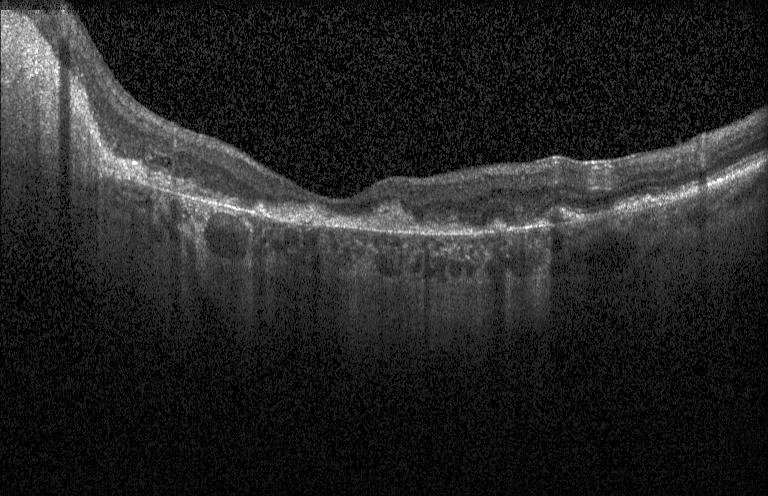
Heidelberg Spectralis OCT system. Macular scan. Spectral-domain optical coherence tomography. Optical coherence tomography scan
Diagnosis: CNV.